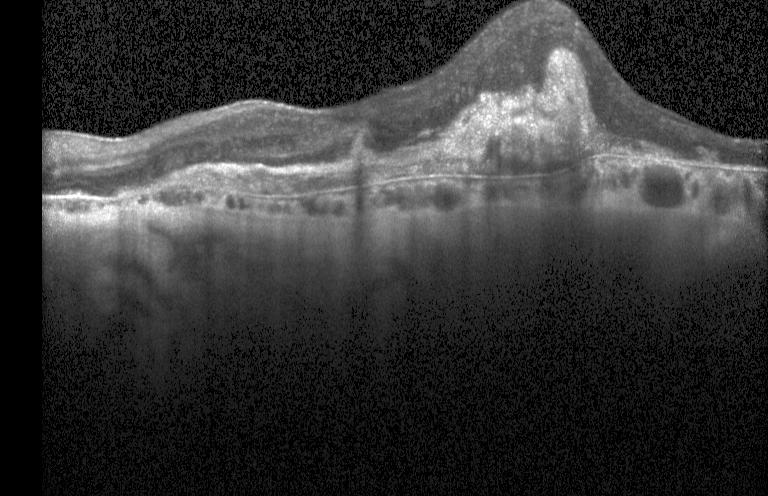 Instrument: Heidelberg Spectralis, optical coherence tomography scan — Impression: choroidal neovascularization (CNV).